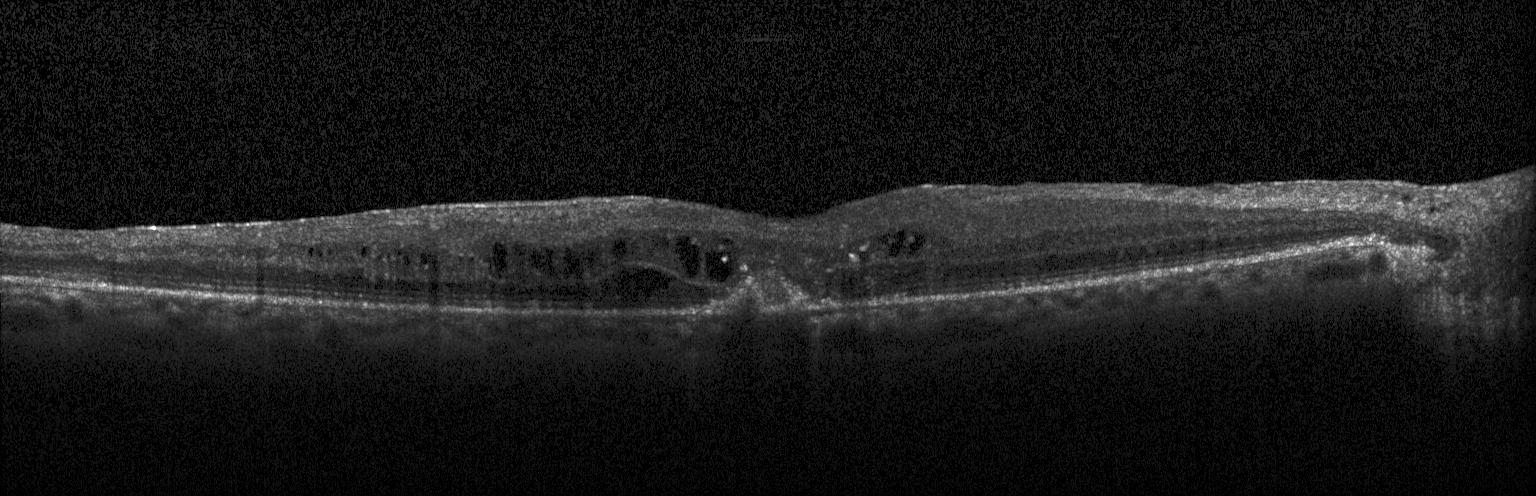

Spectral-domain OCT · OCT B-scan · instrument: Heidelberg Spectralis.
This B-scan demonstrates sub-RPE drusenoid deposits.